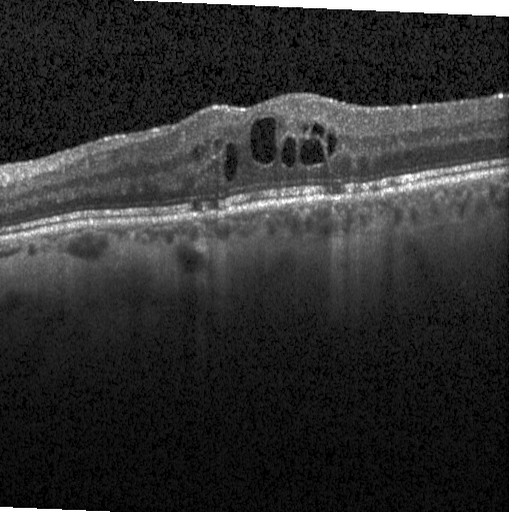
Spectral-domain optical coherence tomography. Centered on the fovea. OCT B-scan. Heidelberg Spectralis. Finding: DME.